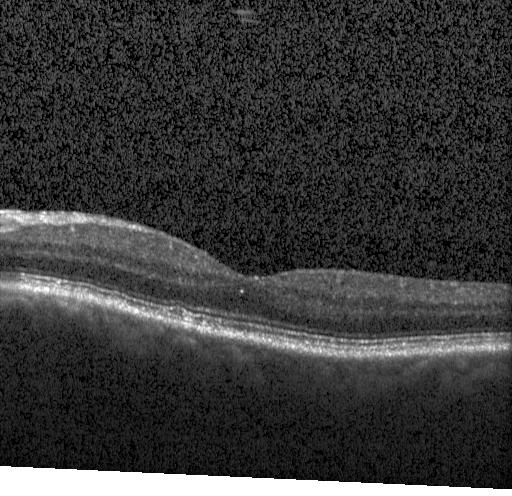 Impression: sub-RPE drusenoid deposits.